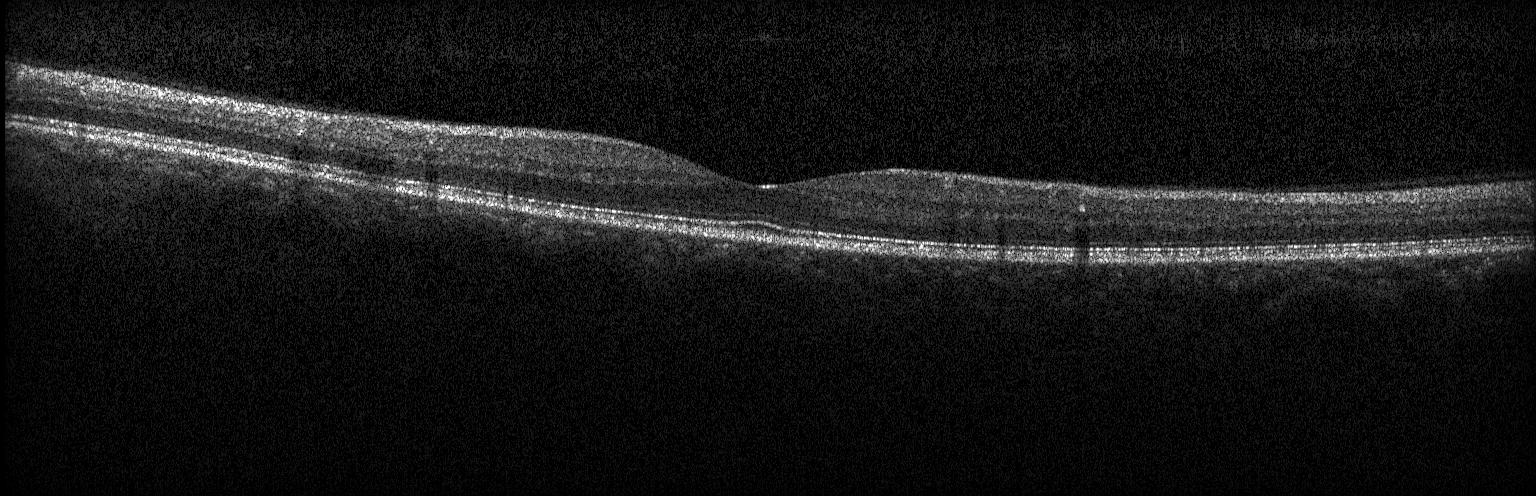 OCT B-scan · acquired on a Heidelberg Spectralis · spectral-domain OCT · fovea-centered.
Dx: neither choroidal neovascularization, diabetic macular edema, nor drusen.